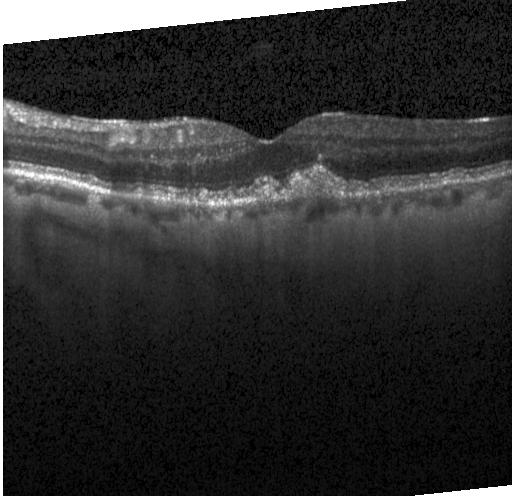
Acquired on a Heidelberg Spectralis. OCT line scan. Macular scan
Impression: multiple drusen.